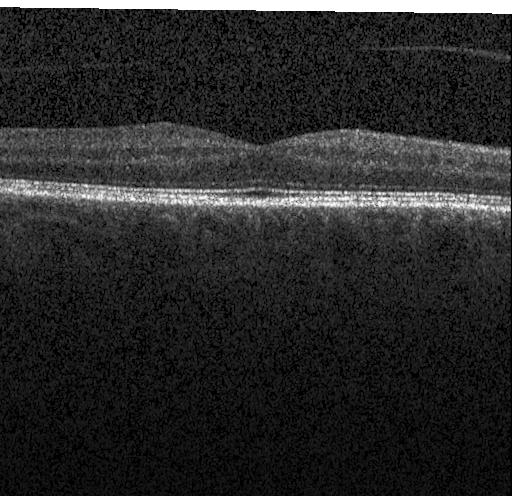

OCT line scan — This B-scan demonstrates no choroidal neovascularization, no diabetic macular edema, and no drusen.